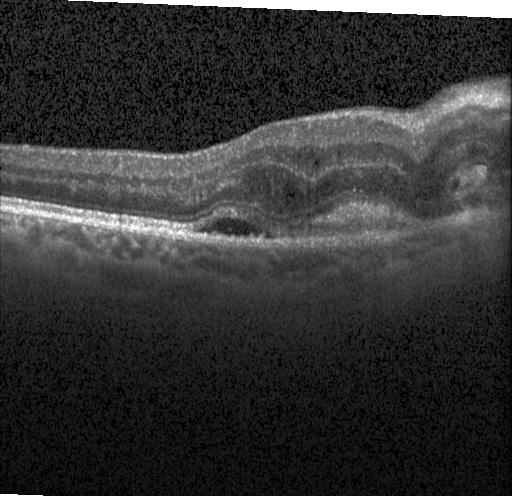

Finding: CNV.